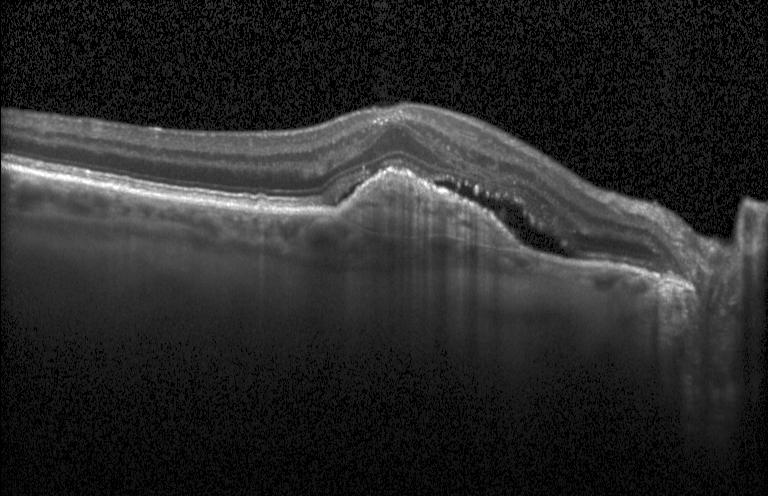 Macular scan · retinal OCT cross-section · Heidelberg Spectralis OCT system. Finding: CNV.